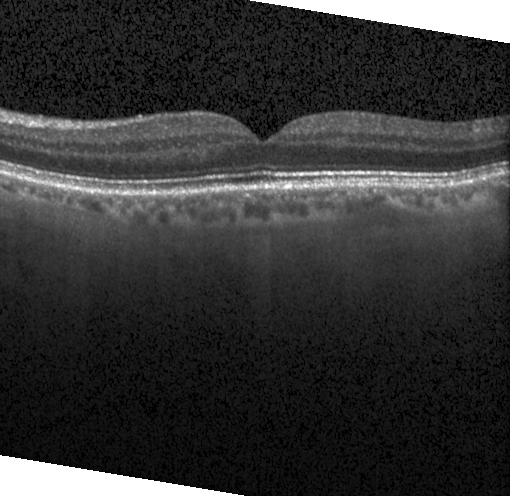 Retinal OCT cross-section · macular scan · SD-OCT · acquired on a Heidelberg Spectralis. Dx: no choroidal neovascularization, no diabetic macular edema, and no drusen.